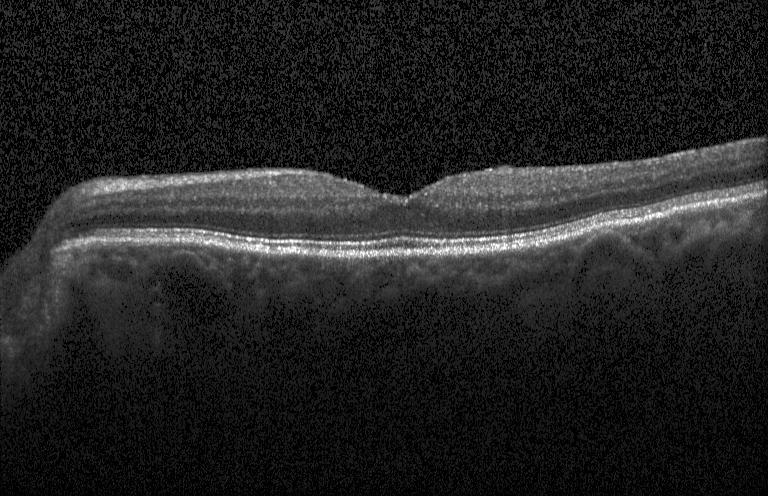
Spectral-domain OCT B-scan: neither choroidal neovascularization, diabetic macular edema, nor drusen.